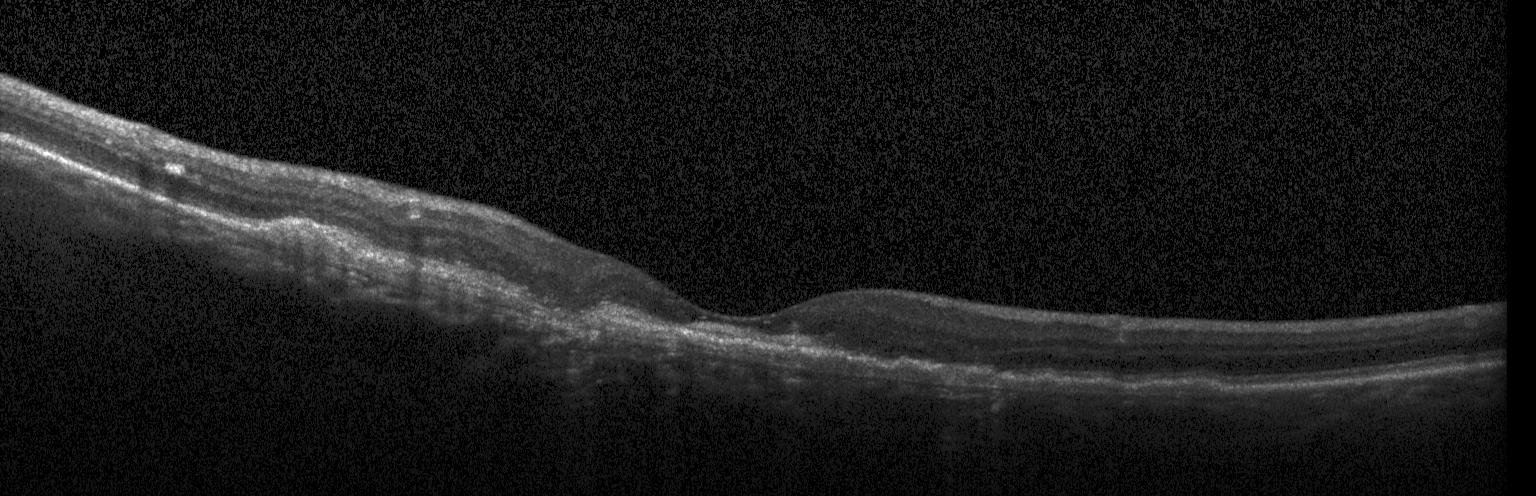
OCT B-scan showing a choroidal neovascular membrane.